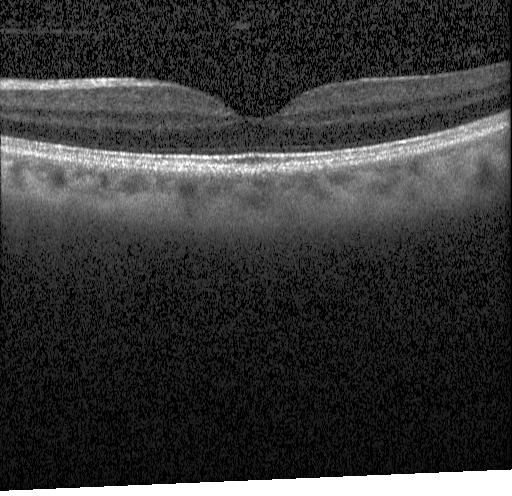 Finding: neither choroidal neovascularization, diabetic macular edema, nor drusen.